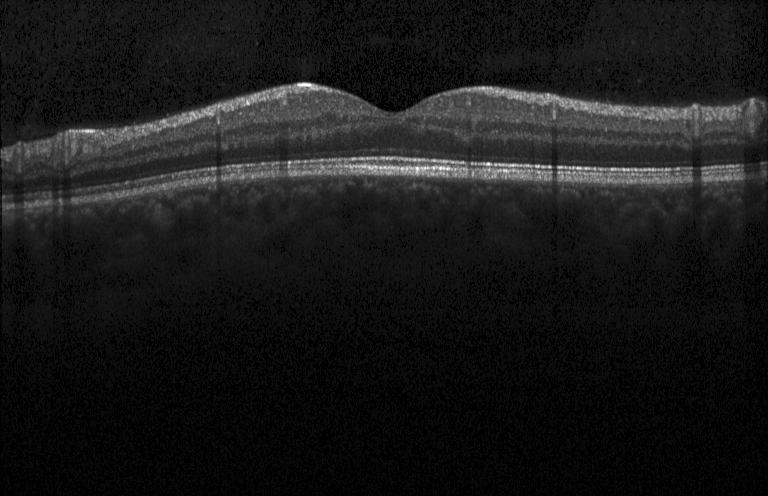

OCT finding: no choroidal neovascularization, diabetic macular edema, or drusen.